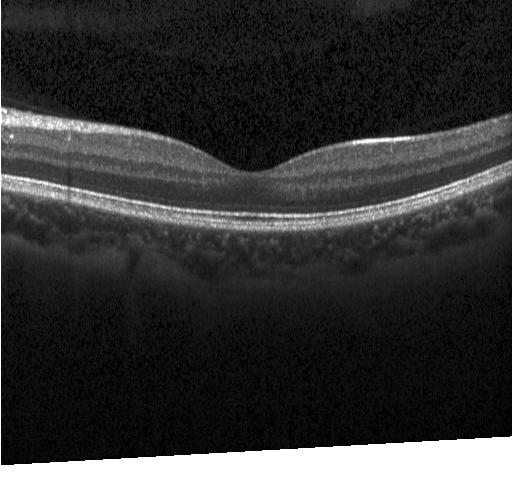
Macular OCT demonstrating no evidence of CNV, DME, or drusen.